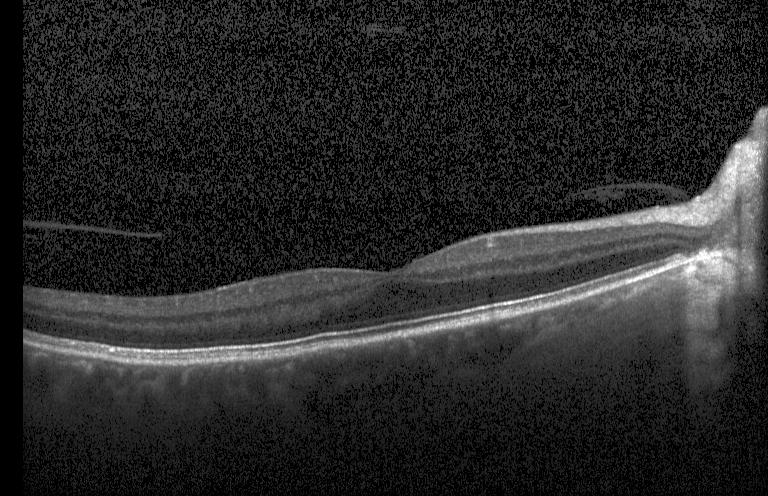 SD-OCT · optical coherence tomography B-scan. Finding: no choroidal neovascularization, no diabetic macular edema, and no drusen.